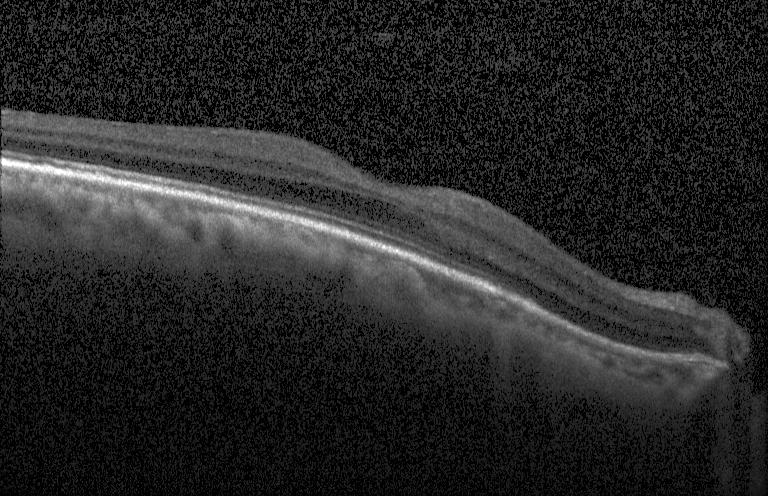
Heidelberg Spectralis OCT system. Retinal OCT cross-section. SD-OCT. Macular scan
Dx: no choroidal neovascularization, diabetic macular edema, or drusen.